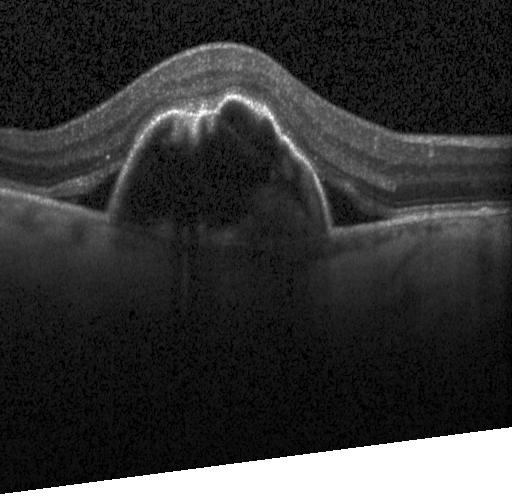
SD-OCT, OCT line scan.
Finding: CNV.